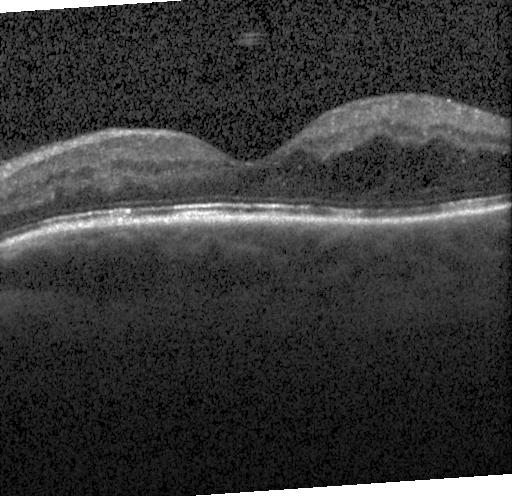

Heidelberg Spectralis. SD-OCT. Optical coherence tomography B-scan. Fovea-centered
Impression: diabetic macular edema.